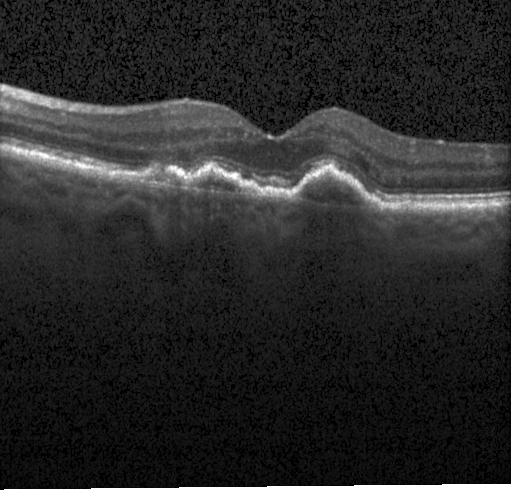
The scan shows a choroidal neovascular membrane.